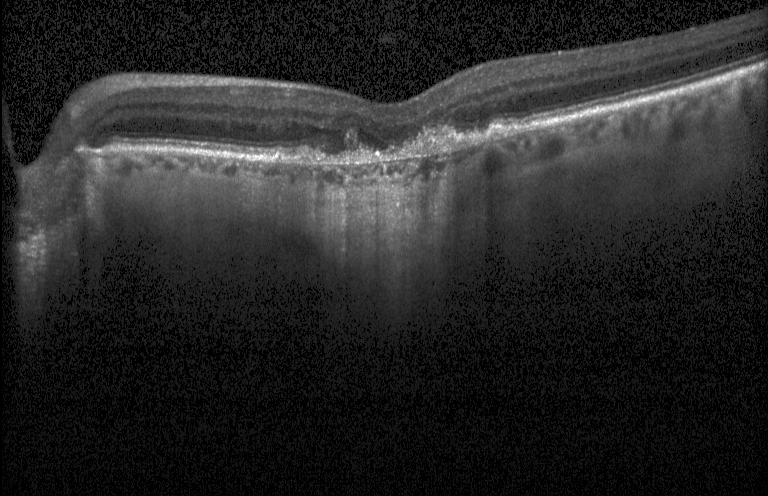
OCT B-scan. Heidelberg Spectralis OCT system. Finding: a choroidal neovascular membrane.